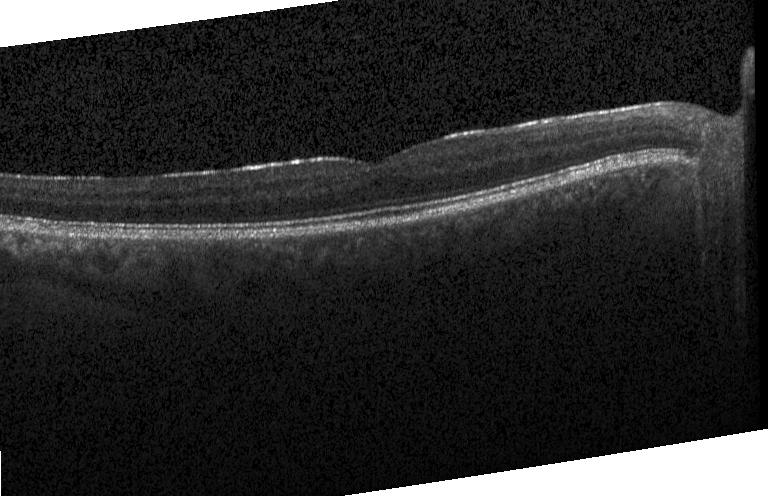
Spectral-domain OCT B-scan: no CNV, no DME, and no drusen.